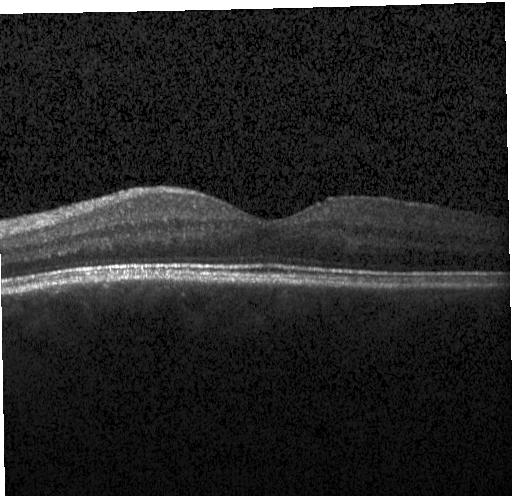 Optical coherence tomography scan. This B-scan demonstrates no choroidal neovascularization, diabetic macular edema, or drusen.